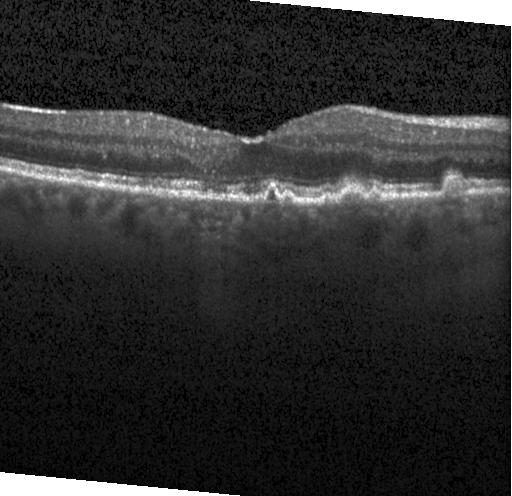
Retinal OCT cross-section. Finding: sub-RPE drusenoid deposits.